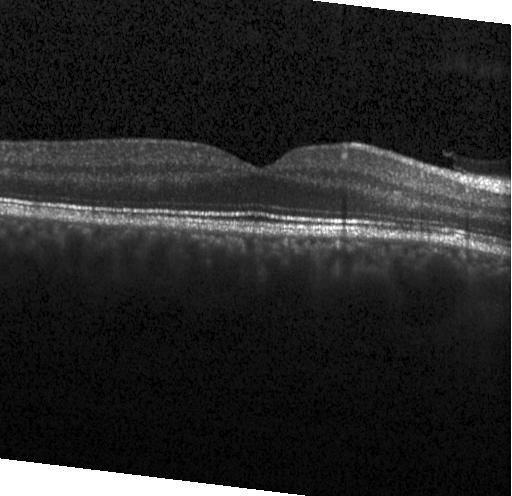
Retinal OCT B-scan.
Impression: no choroidal neovascularization, diabetic macular edema, or drusen.